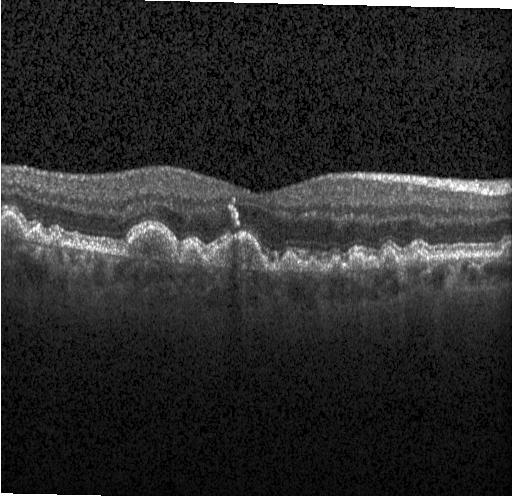
Assessment: sub-RPE drusenoid deposits.